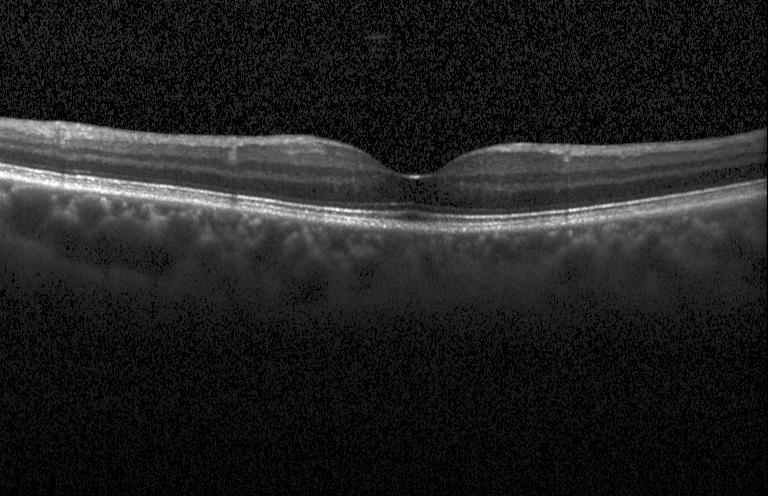
OCT scan showing neither choroidal neovascularization, diabetic macular edema, nor drusen.